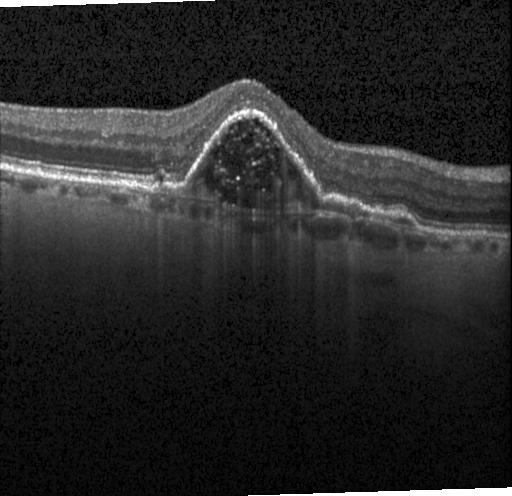
Diagnosis: choroidal neovascularization.